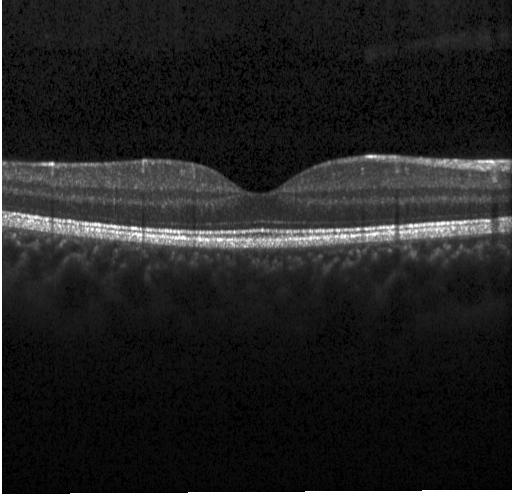

Finding: no evidence of choroidal neovascularization, diabetic macular edema, or drusen.